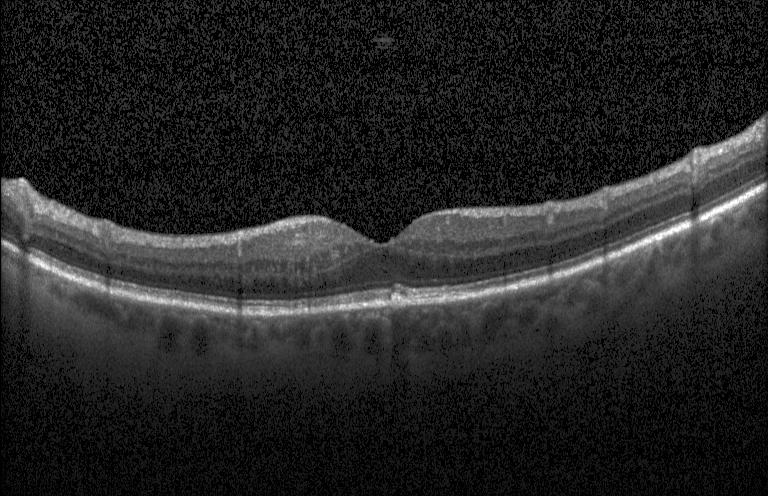

Dx: sub-RPE drusenoid deposits.